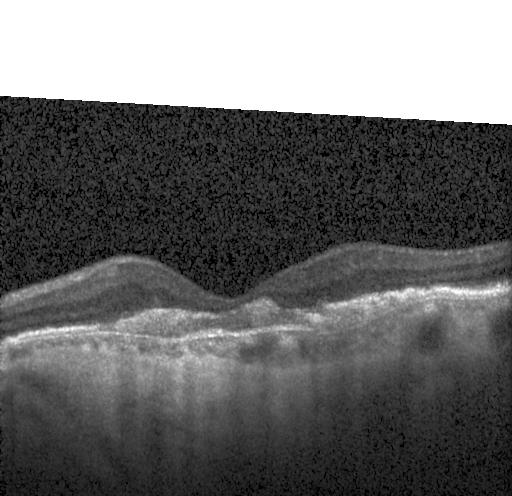 Impression: a choroidal neovascular membrane.